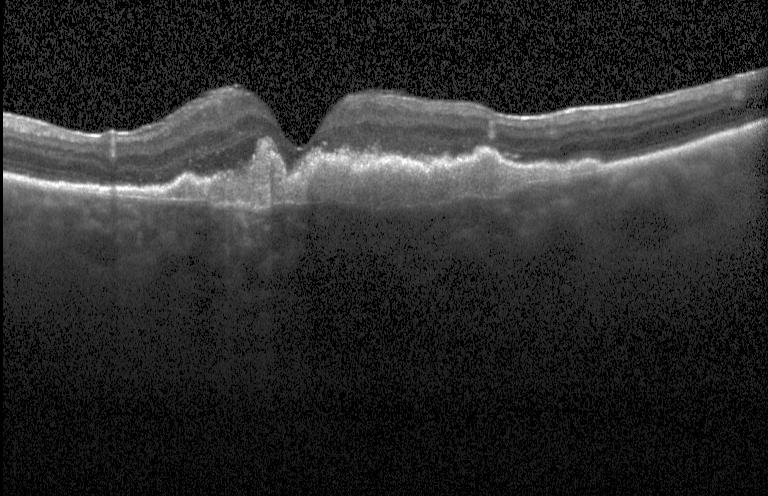

Spectral-domain OCT B-scan: CNV.